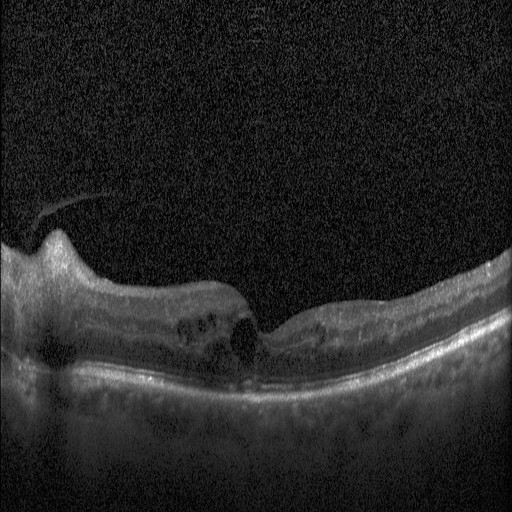 Spectral-domain optical coherence tomography. Optical coherence tomography B-scan. Centered on the fovea. Dx: diabetic macular edema.